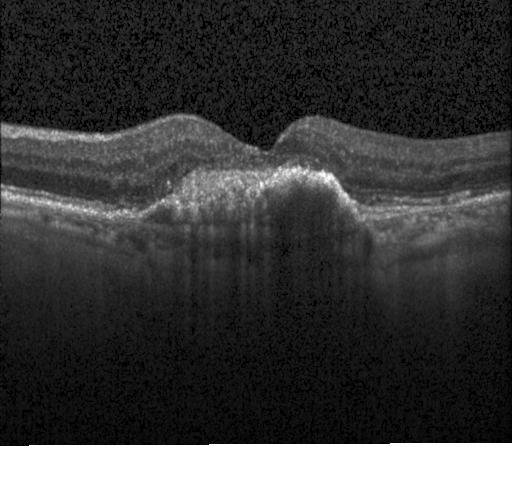 Heidelberg Spectralis. Centered on the fovea. OCT line scan — Macular OCT: choroidal neovascularization.